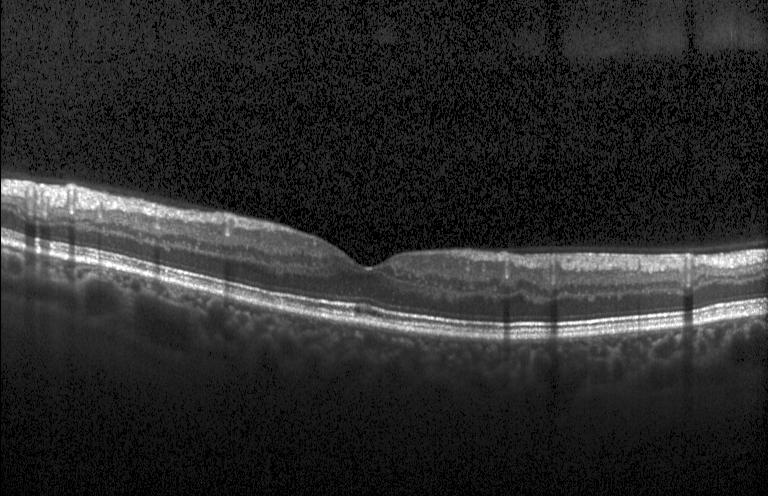 OCT scan showing no CNV, DME, or drusen.